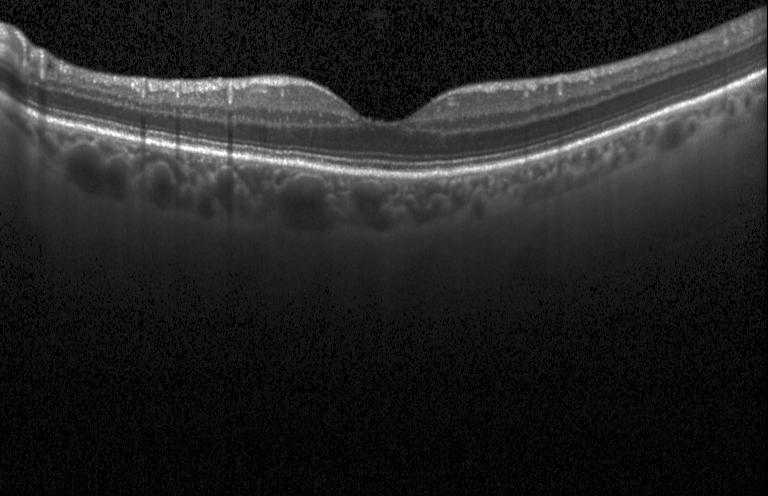

Horizontal scan through the fovea. Optical coherence tomography scan. Instrument: Heidelberg Spectralis.
Finding: neither CNV, DME, nor drusen.